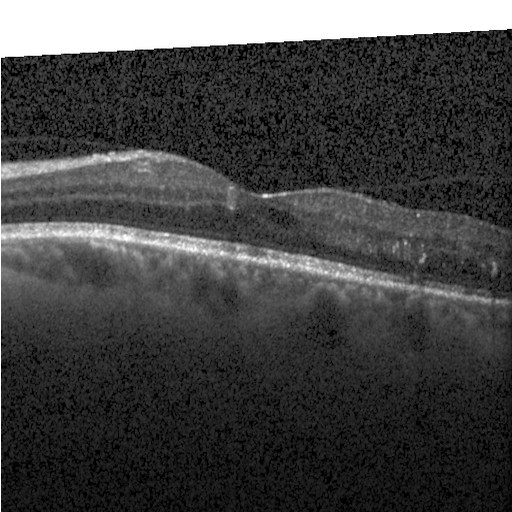

Optical coherence tomography B-scan. Horizontal scan through the fovea. SD-OCT.
This B-scan demonstrates diabetic macular edema (DME).